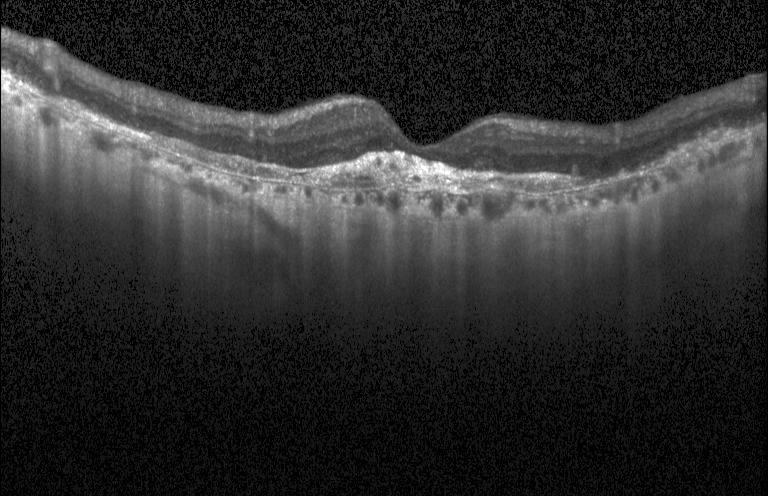
This B-scan demonstrates a choroidal neovascular membrane.